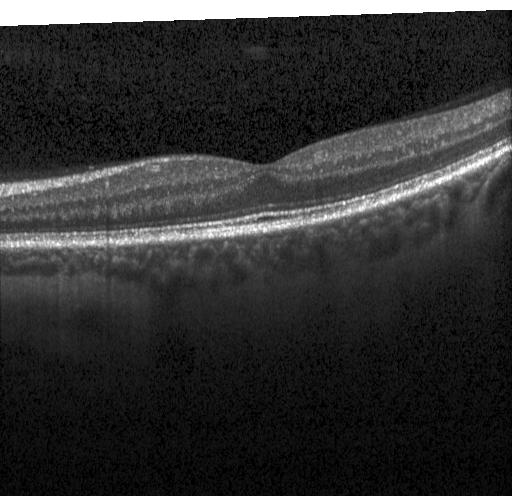
Macular scan, retinal OCT cross-section — Impression: no evidence of CNV, DME, or drusen.